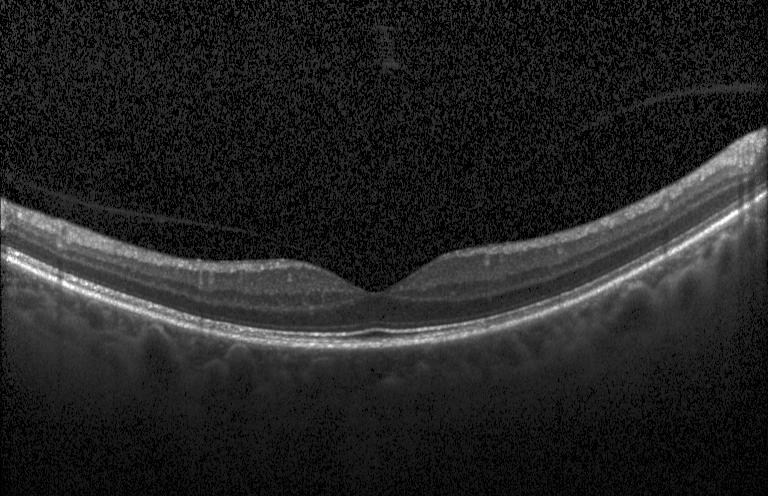

Fovea-centered · OCT line scan — Diagnosis: neither choroidal neovascularization, diabetic macular edema, nor drusen.